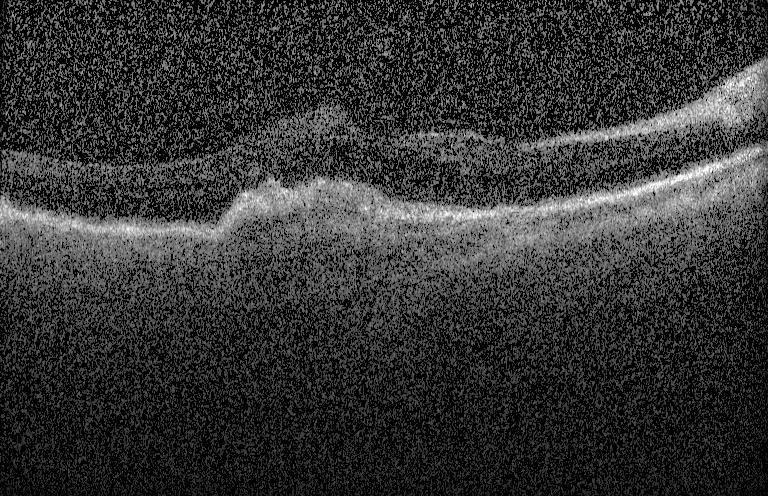
OCT B-scan; fovea-centered
Dx: choroidal neovascularization.